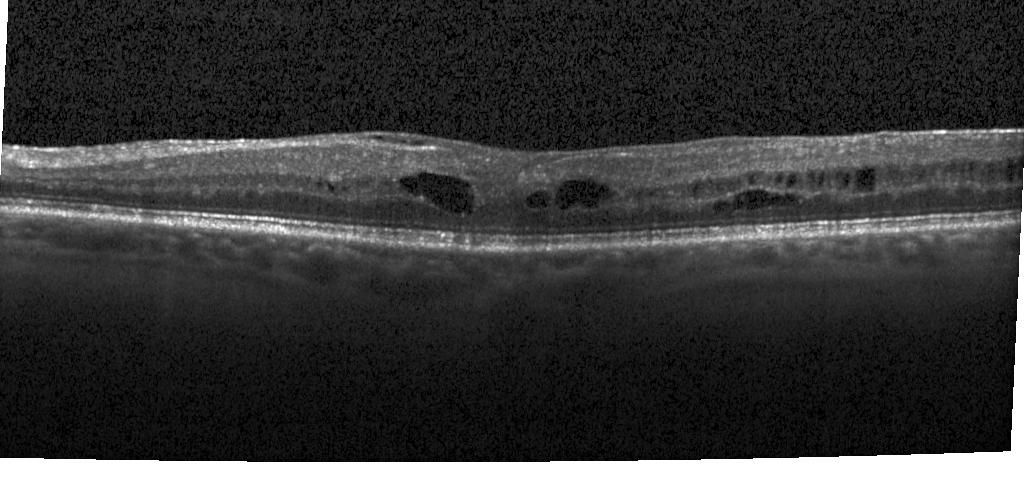
Diagnosis: diabetic macular edema.